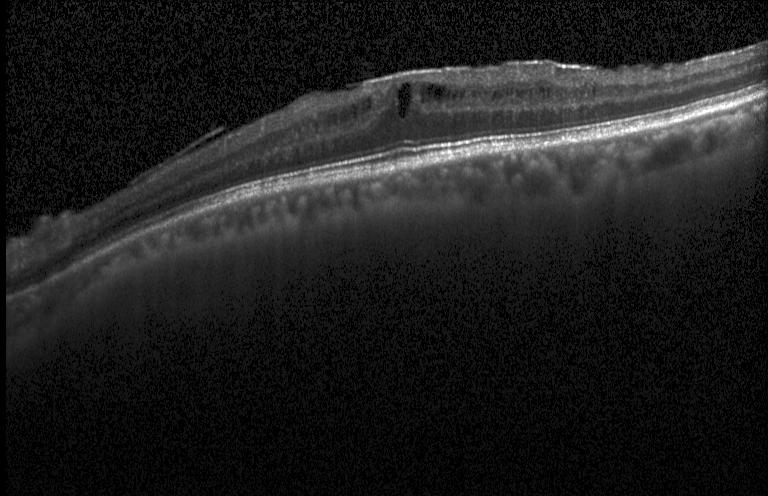

Retinal OCT cross-section; Heidelberg Spectralis OCT system
The scan shows diabetic macular edema (DME).